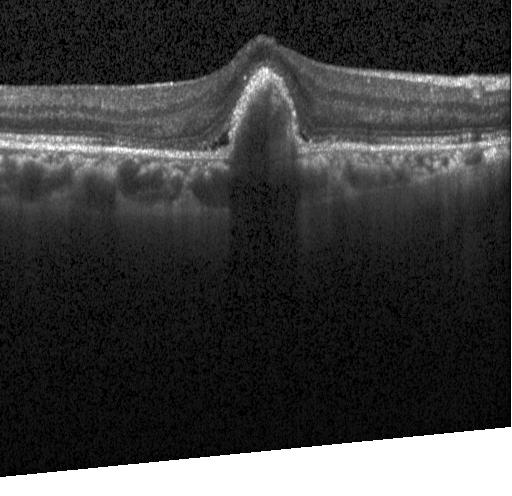 This B-scan demonstrates a choroidal neovascular membrane.